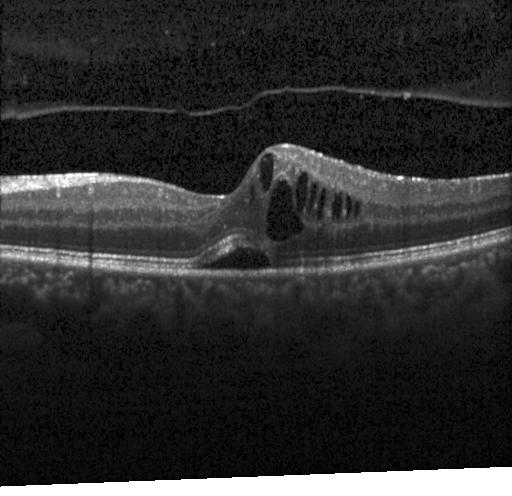
Retinal OCT B-scan.
Finding: diabetic macular edema (DME).